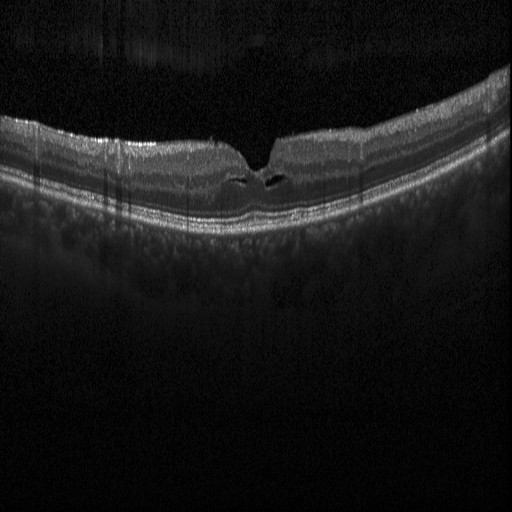
Finding: DME.